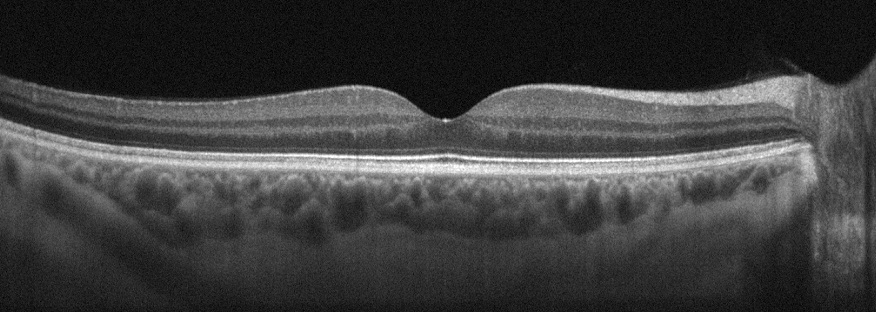

OCT line scan. Acquired on an Optovue Avanti RTVue XR. Macular OCT: absence of AMD, DME, ERM, RAO, RVO, and vitreomacular interface disease.